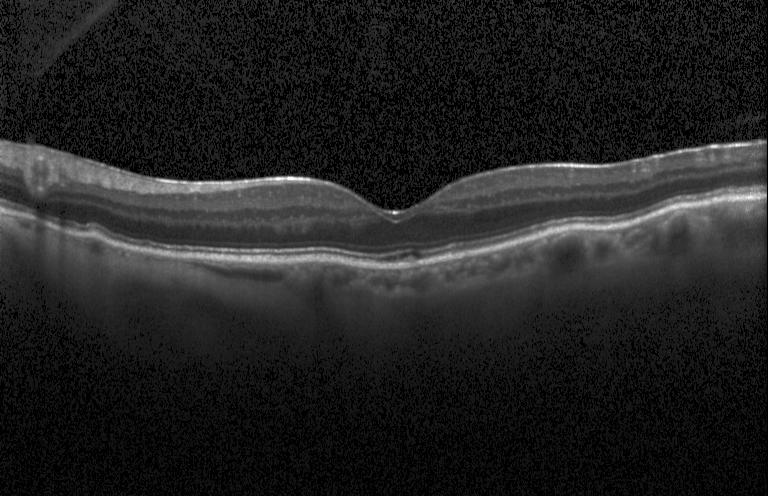 Fovea-centered. Optical coherence tomography B-scan.
No choroidal neovascularization, no diabetic macular edema, and no drusen.